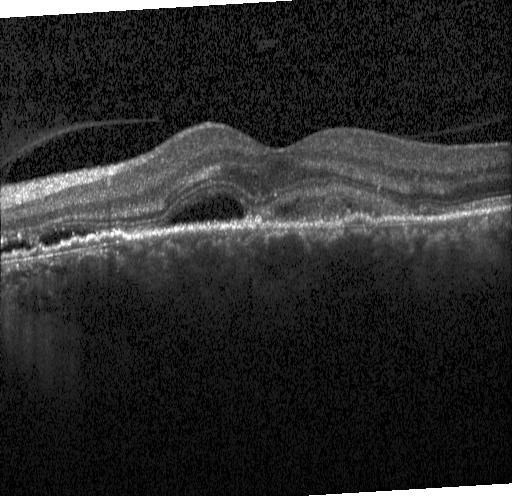
Dx: CNV.